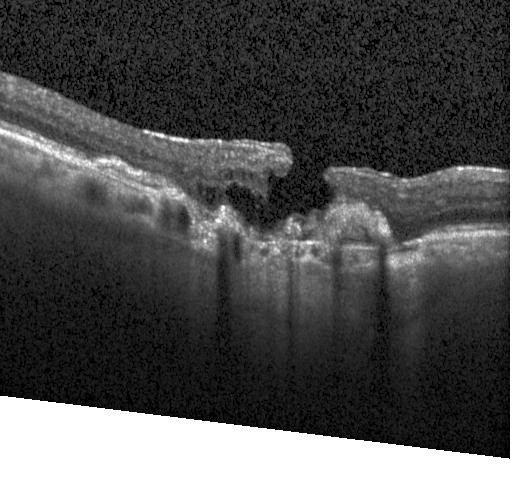

Spectral-domain OCT B-scan: a choroidal neovascular membrane.